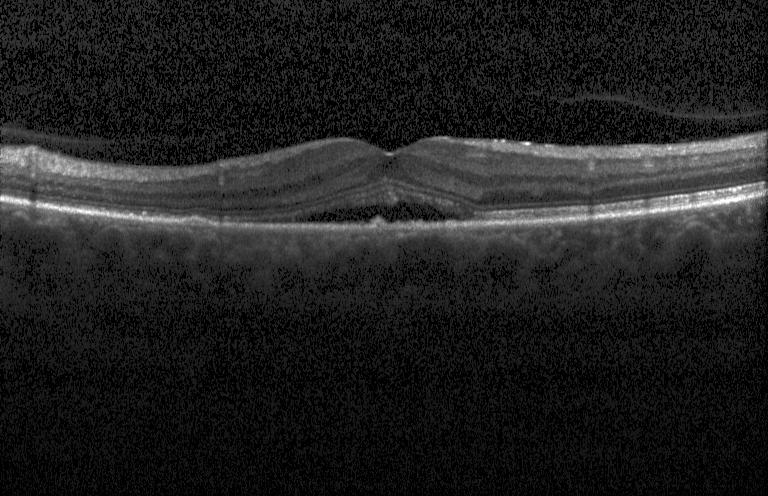

Retinal OCT cross-section — Diagnosis: a choroidal neovascular membrane.